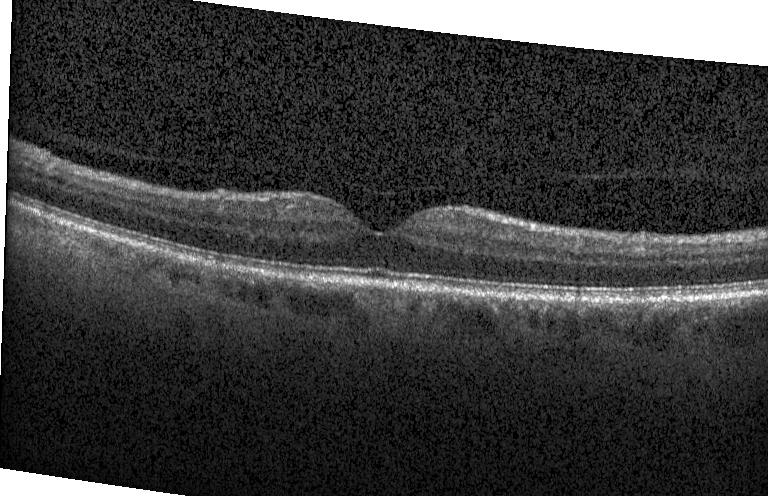
Diagnosis: no choroidal neovascularization, no diabetic macular edema, and no drusen.